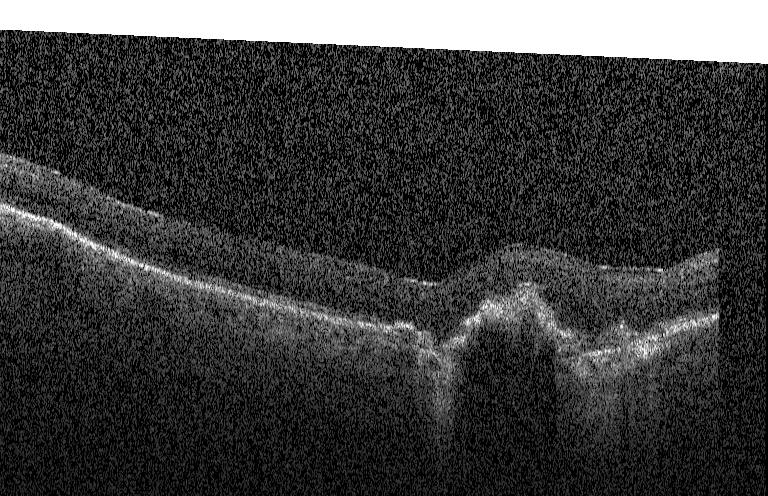

Diagnosis: a choroidal neovascular membrane.